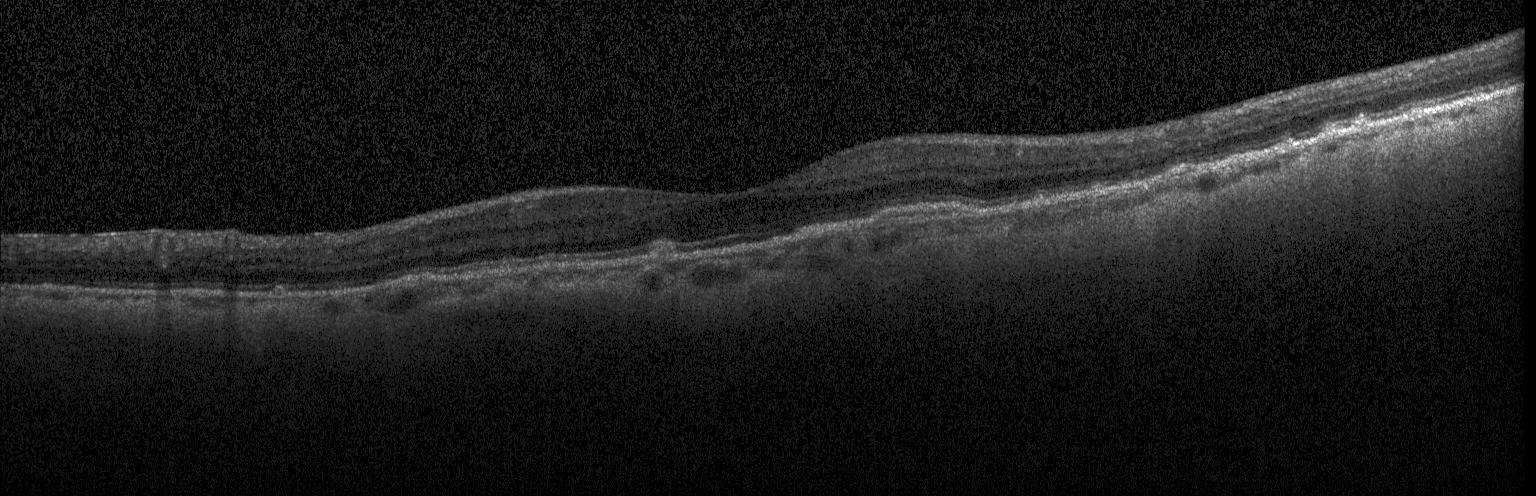

Macular OCT demonstrating sub-RPE drusenoid deposits.